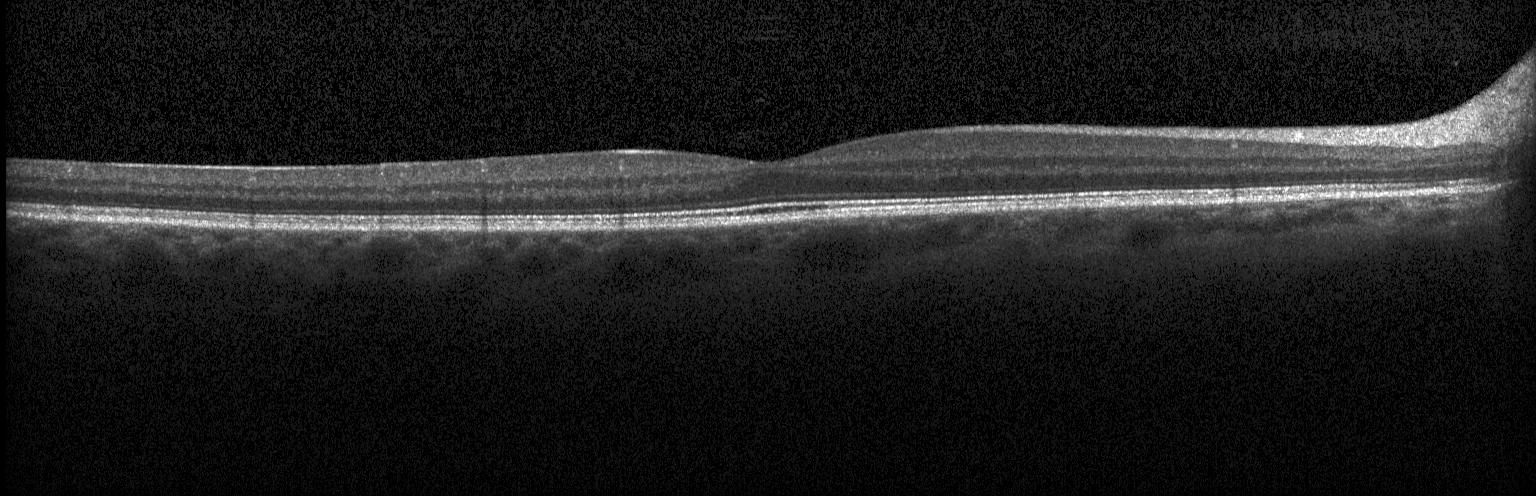 Fovea-centered; OCT B-scan. Diagnosis: neither CNV, DME, nor drusen.